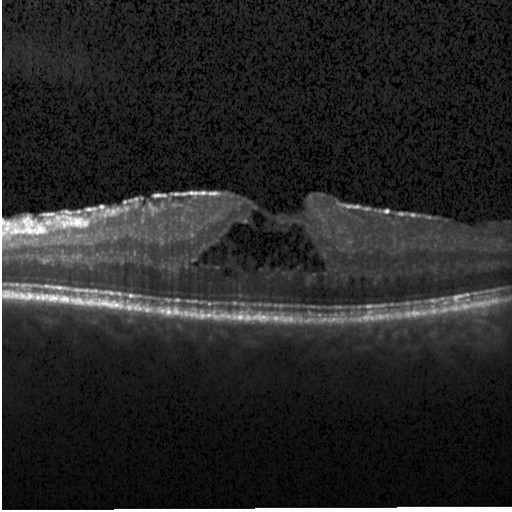 Centered on the fovea · Heidelberg Spectralis · retinal OCT B-scan · SD-OCT — Assessment: DME.